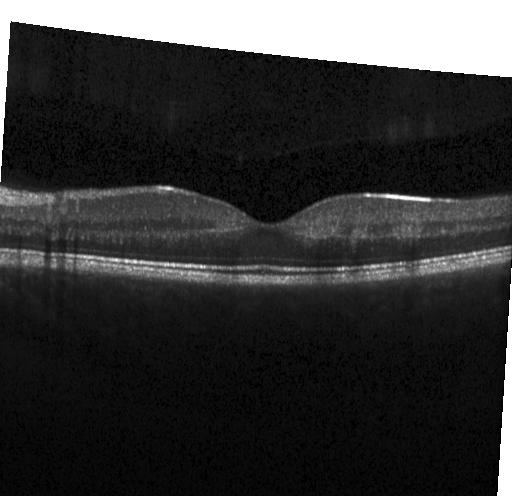

Optical coherence tomography B-scan; spectral-domain OCT.
Macular OCT: no choroidal neovascularization, diabetic macular edema, or drusen.